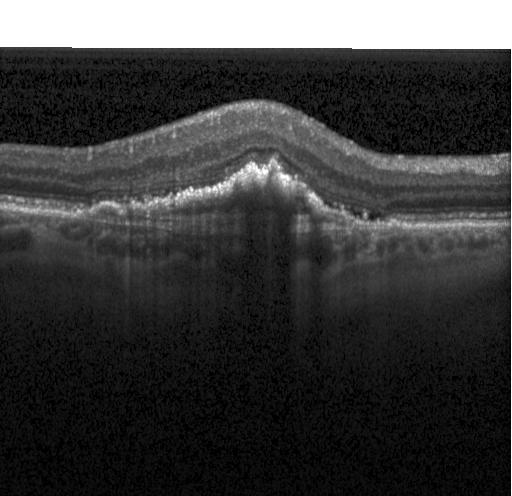 Instrument: Heidelberg Spectralis · macular scan · OCT line scan · spectral-domain OCT — This B-scan demonstrates a choroidal neovascular membrane.